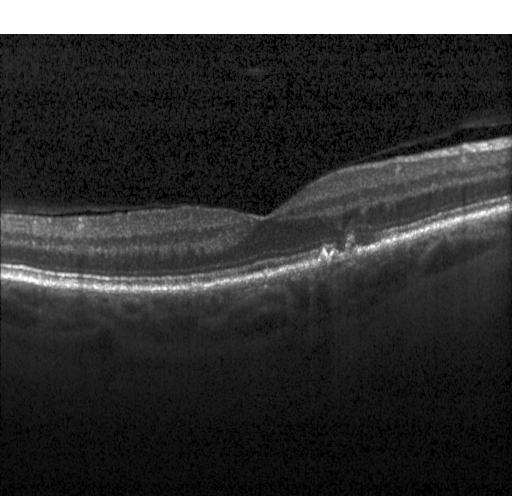 Retinal OCT B-scan — Dx: multiple drusen.